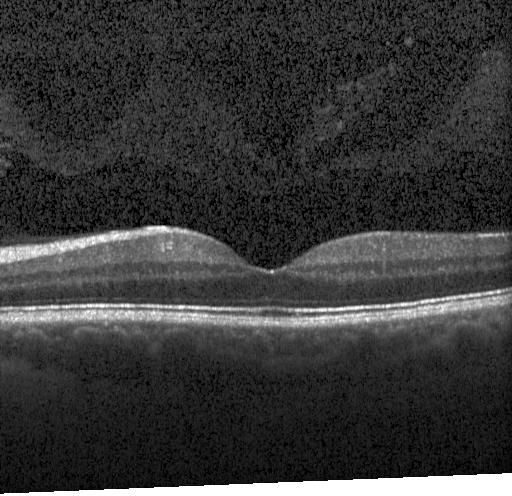

Optical coherence tomography B-scan, Heidelberg Spectralis, fovea-centered
Macular OCT: neither choroidal neovascularization, diabetic macular edema, nor drusen.